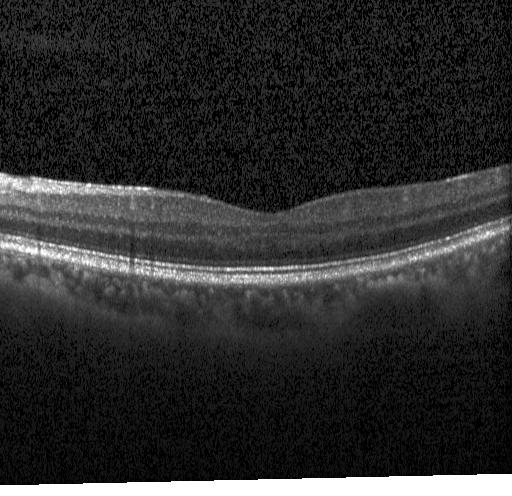
Finding: neither choroidal neovascularization, diabetic macular edema, nor drusen.